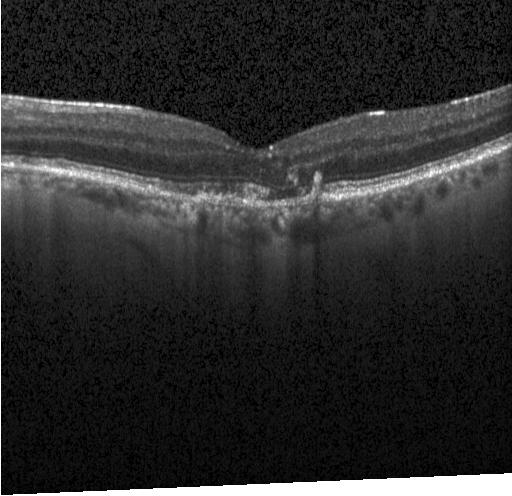 Diagnosis: choroidal neovascularization (CNV).